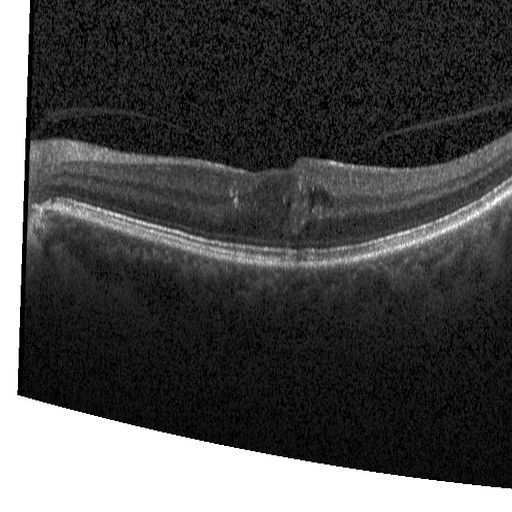

OCT B-scan showing DME.